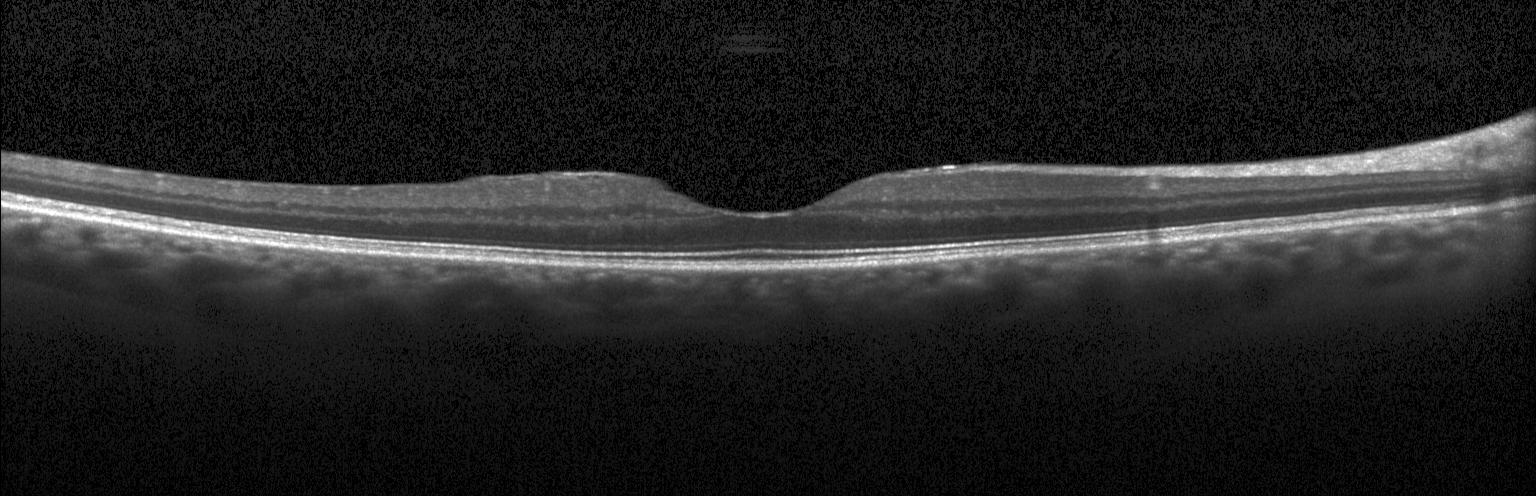
OCT B-scan; macular scan — Finding: no choroidal neovascularization, diabetic macular edema, or drusen.